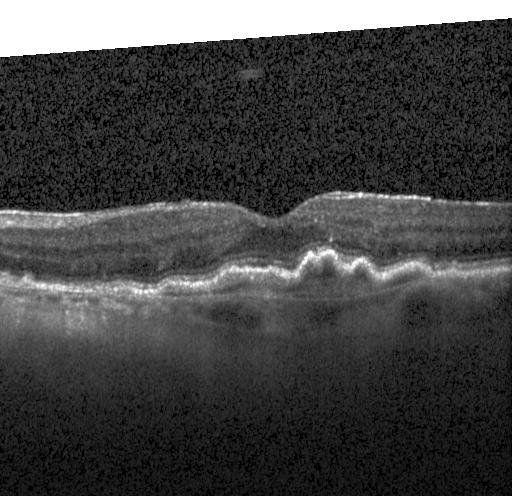
Optical coherence tomography scan; spectral-domain OCT. Finding: choroidal neovascularization (CNV).